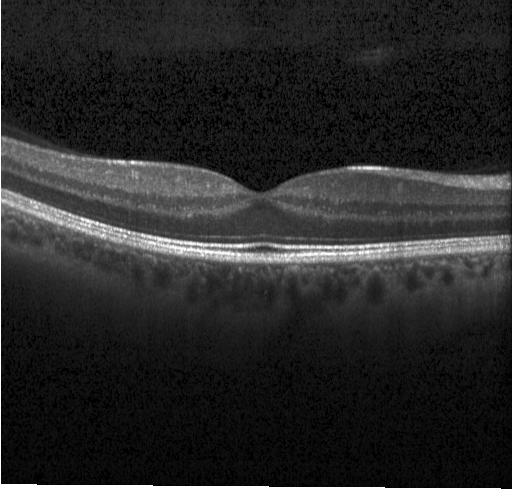

Impression: no choroidal neovascularization, diabetic macular edema, or drusen.